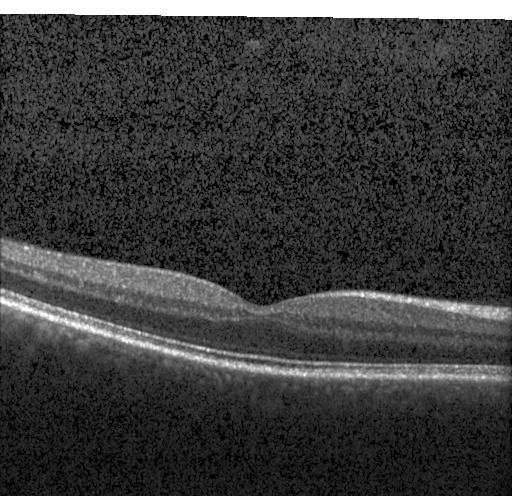

Centered on the fovea · Heidelberg Spectralis OCT system · optical coherence tomography scan.
Diagnosis: no evidence of CNV, DME, or drusen.